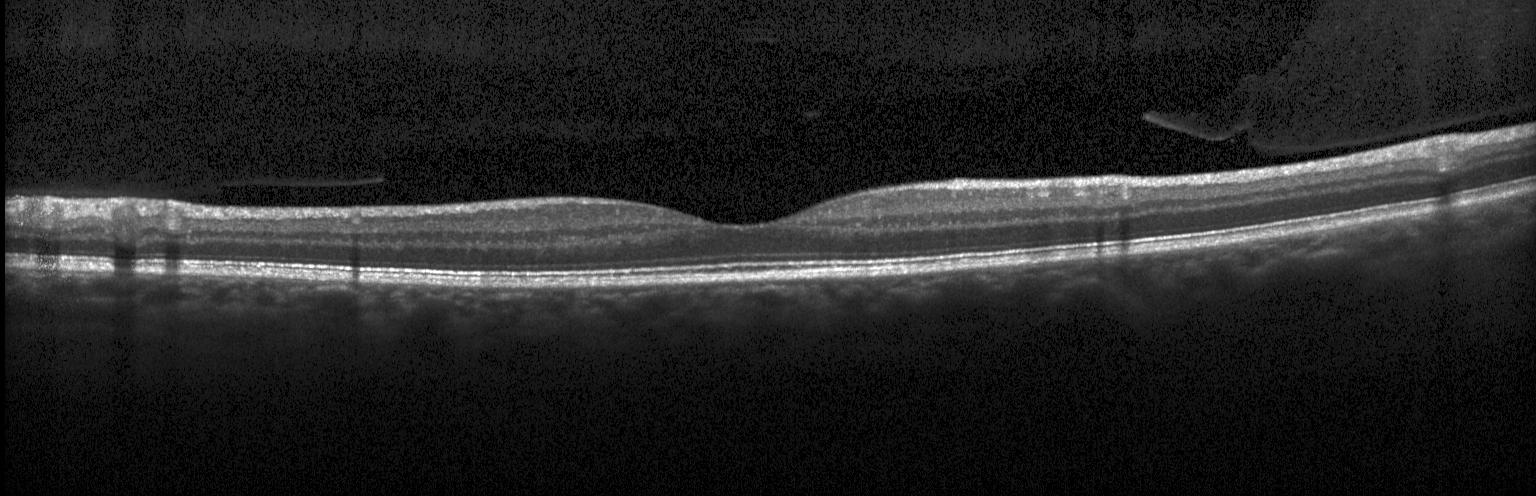
OCT line scan. SD-OCT. Acquired on a Heidelberg Spectralis. Horizontal scan through the fovea
Macular OCT: no choroidal neovascularization, diabetic macular edema, or drusen.